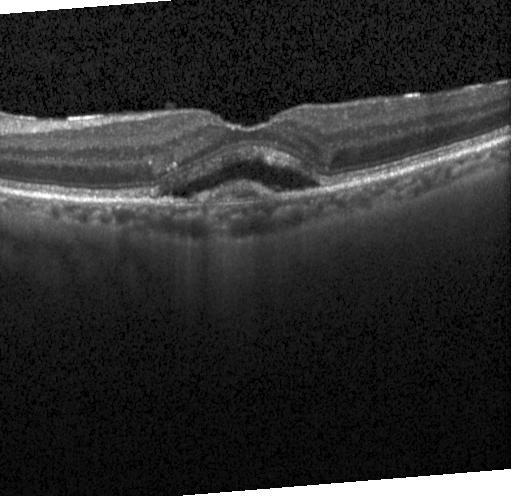 Spectral-domain OCT · retinal OCT B-scan · centered on the fovea.
Assessment: choroidal neovascularization (CNV).